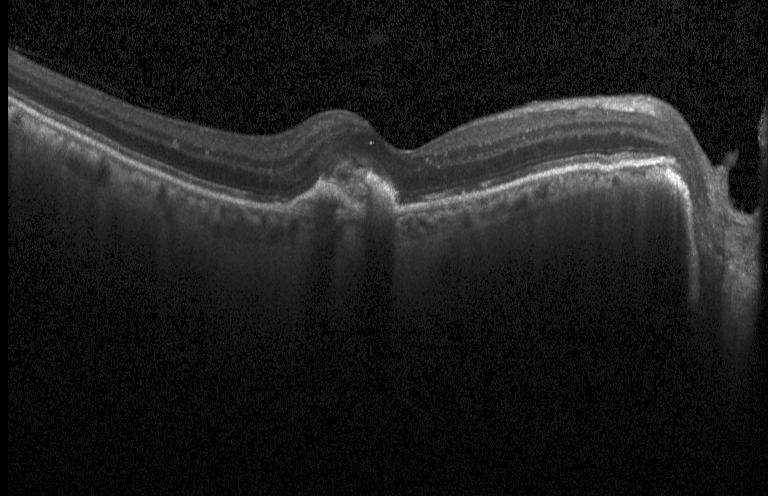
OCT scan showing choroidal neovascularization.